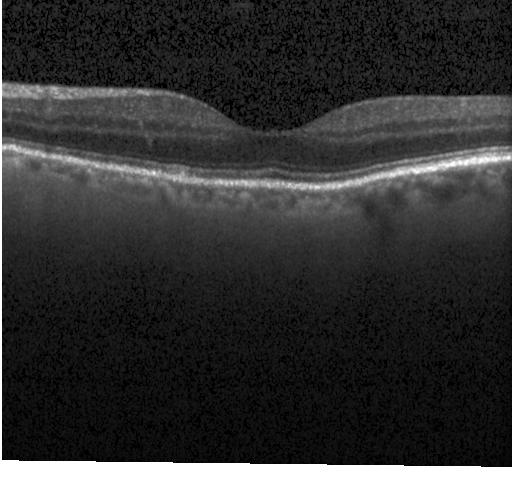

Retinal OCT B-scan · spectral-domain optical coherence tomography. Macular OCT: no evidence of CNV, DME, or drusen.